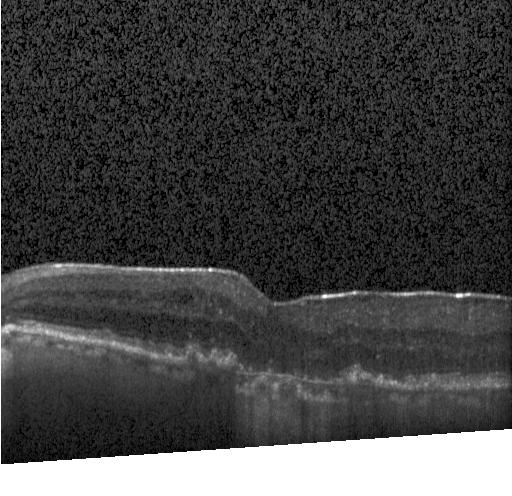 Spectral-domain OCT, retinal OCT B-scan.
This B-scan demonstrates CNV.